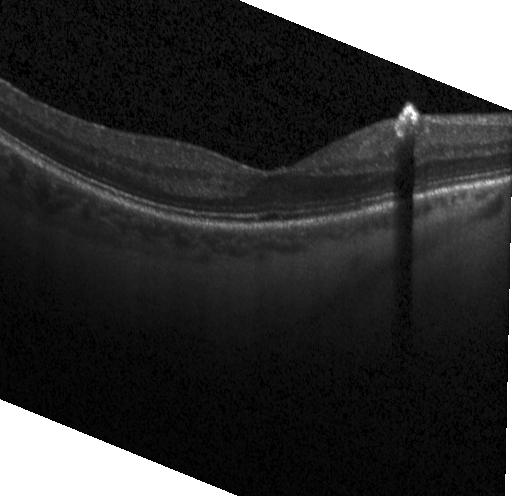
Diagnosis: no choroidal neovascularization, diabetic macular edema, or drusen.